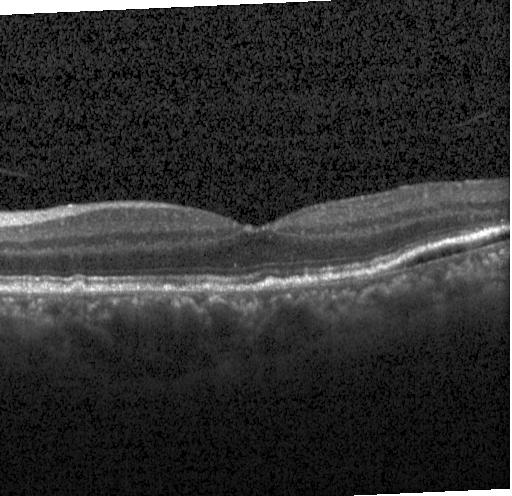 Horizontal scan through the fovea · instrument: Heidelberg Spectralis · SD-OCT · retinal OCT B-scan — Diagnosis: choroidal neovascularization.